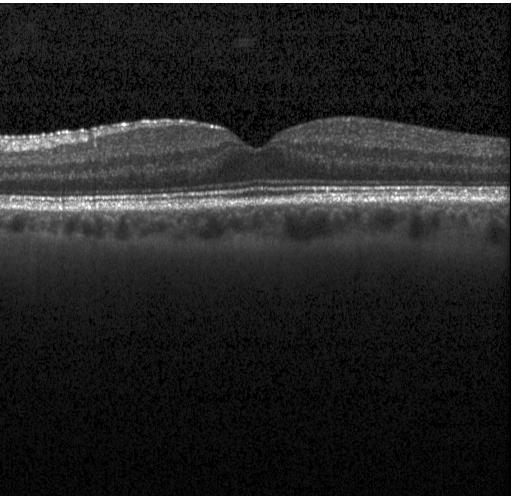 Optical coherence tomography scan.
Impression: no evidence of CNV, DME, or drusen.